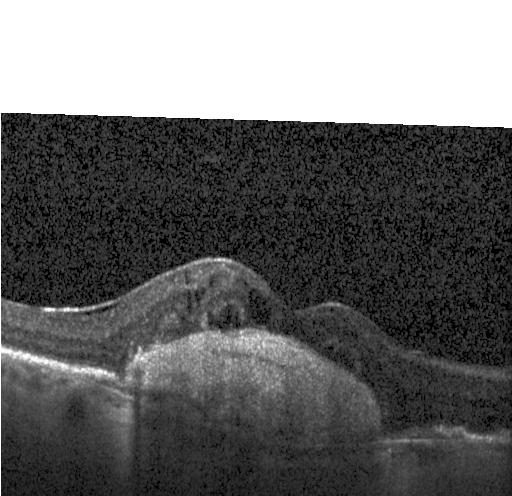 Retinal OCT cross-section. Dx: choroidal neovascularization (CNV).